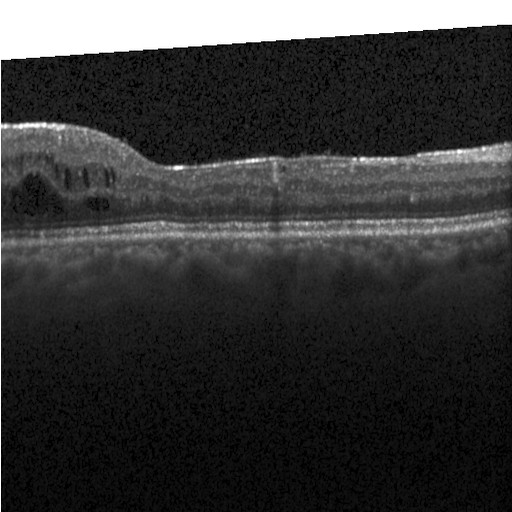

Fovea-centered · acquired on a Heidelberg Spectralis · spectral-domain optical coherence tomography · optical coherence tomography scan
Impression: diabetic macular edema.